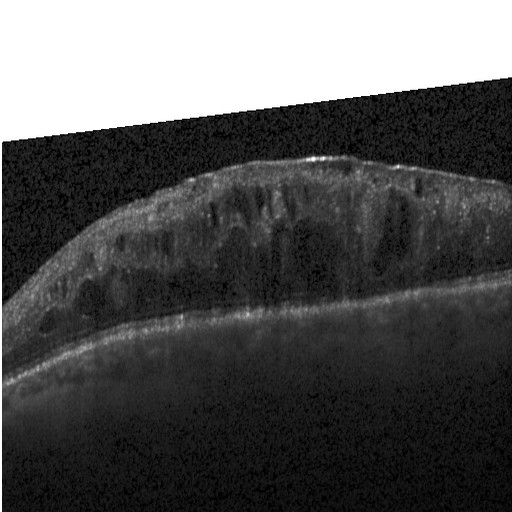 Retinal OCT cross-section showing diabetic macular edema.